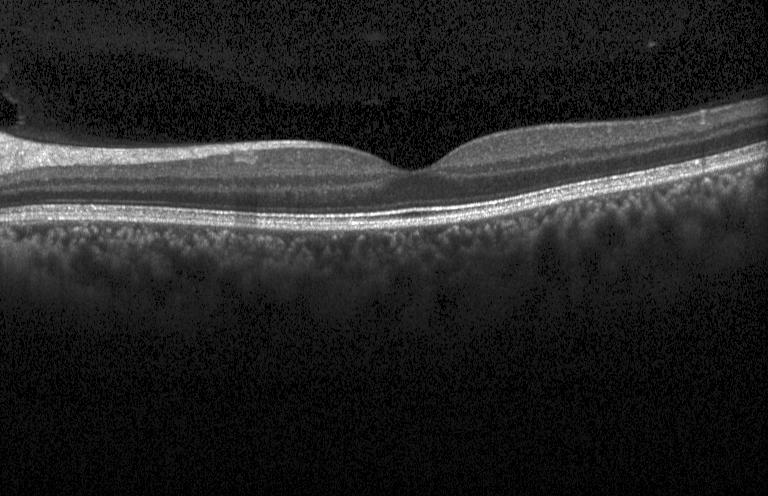

Retinal OCT cross-section showing no choroidal neovascularization, no diabetic macular edema, and no drusen.